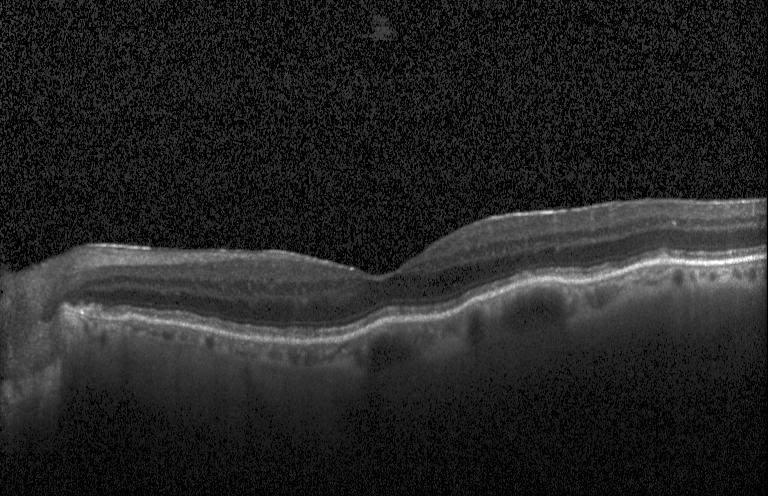
Retinal OCT B-scan, Heidelberg Spectralis — Impression: no choroidal neovascularization, no diabetic macular edema, and no drusen.